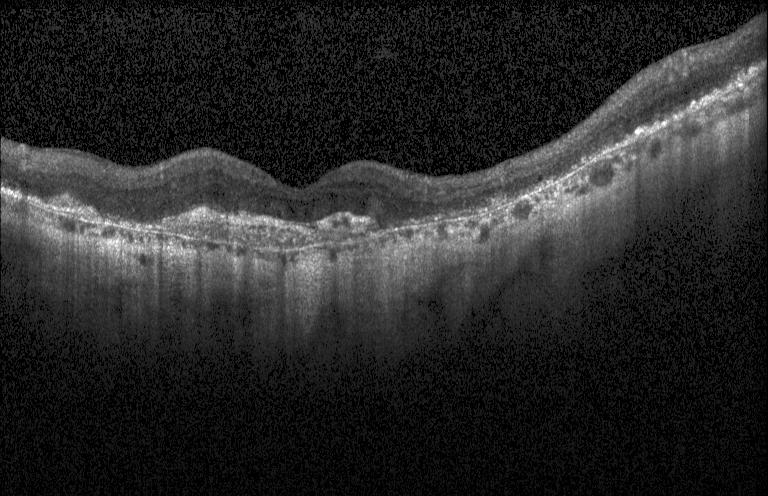 OCT B-scan; centered on the fovea; spectral-domain OCT; acquired on a Heidelberg Spectralis. Dx: CNV.